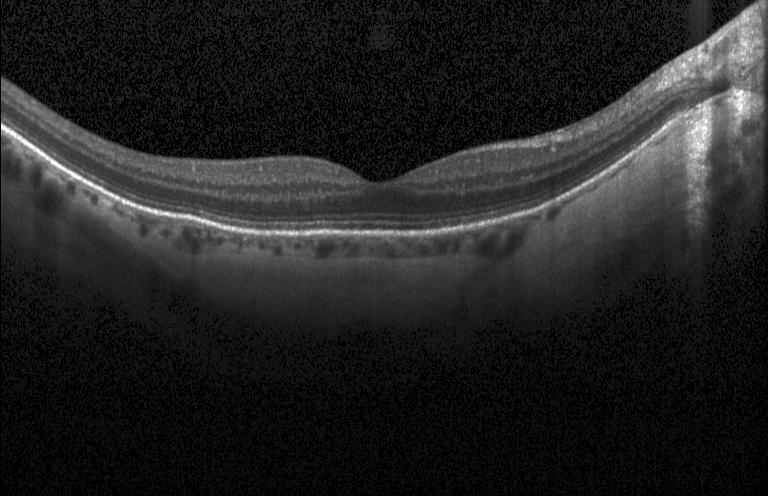 Retinal OCT cross-section — Diagnosis: no evidence of CNV, DME, or drusen.